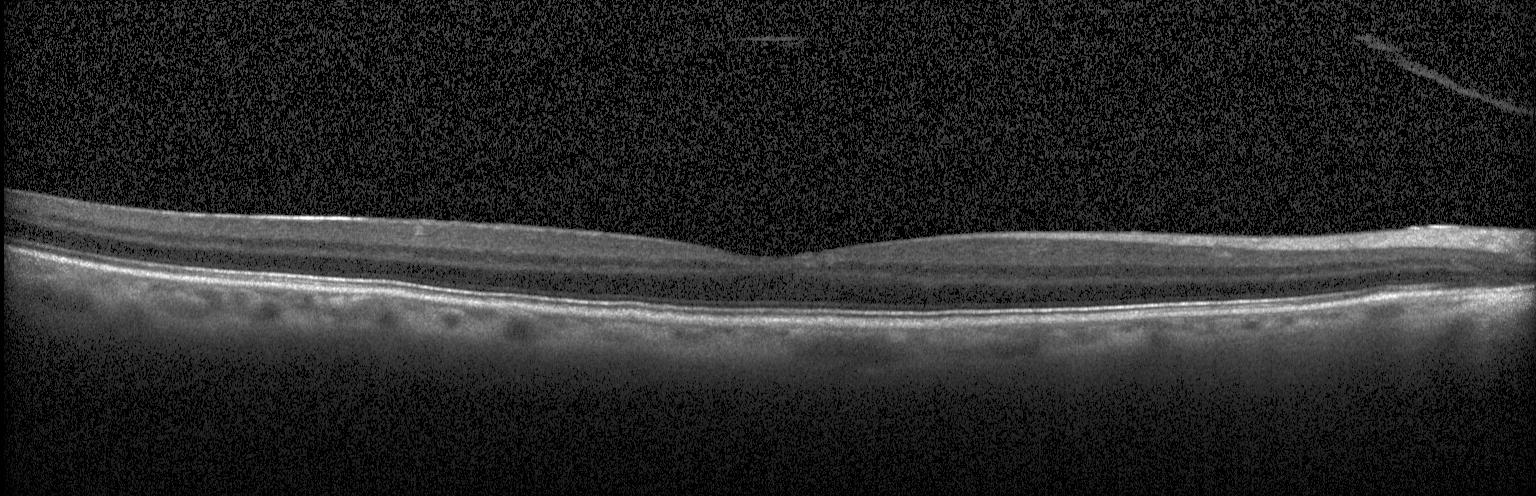

Instrument: Heidelberg Spectralis. Optical coherence tomography B-scan. Centered on the fovea. Dx: neither CNV, DME, nor drusen.